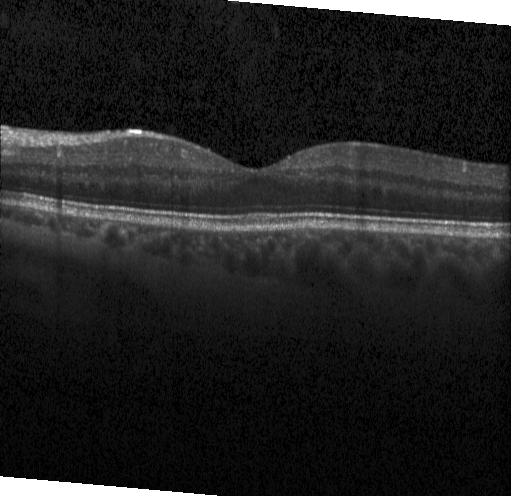 Macular scan. Acquired on a Heidelberg Spectralis. Retinal OCT cross-section. SD-OCT — Impression: no choroidal neovascularization, diabetic macular edema, or drusen.